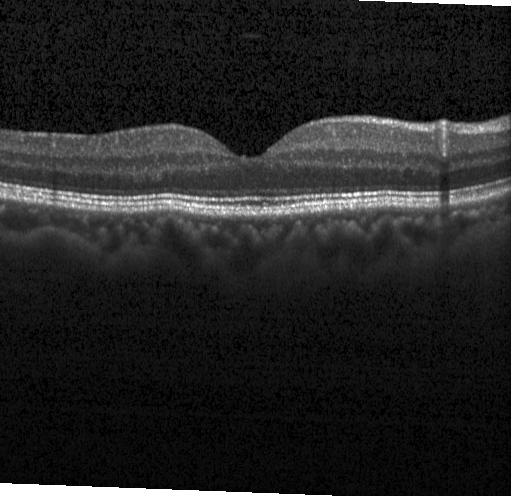

Diagnosis: no CNV, no DME, and no drusen.